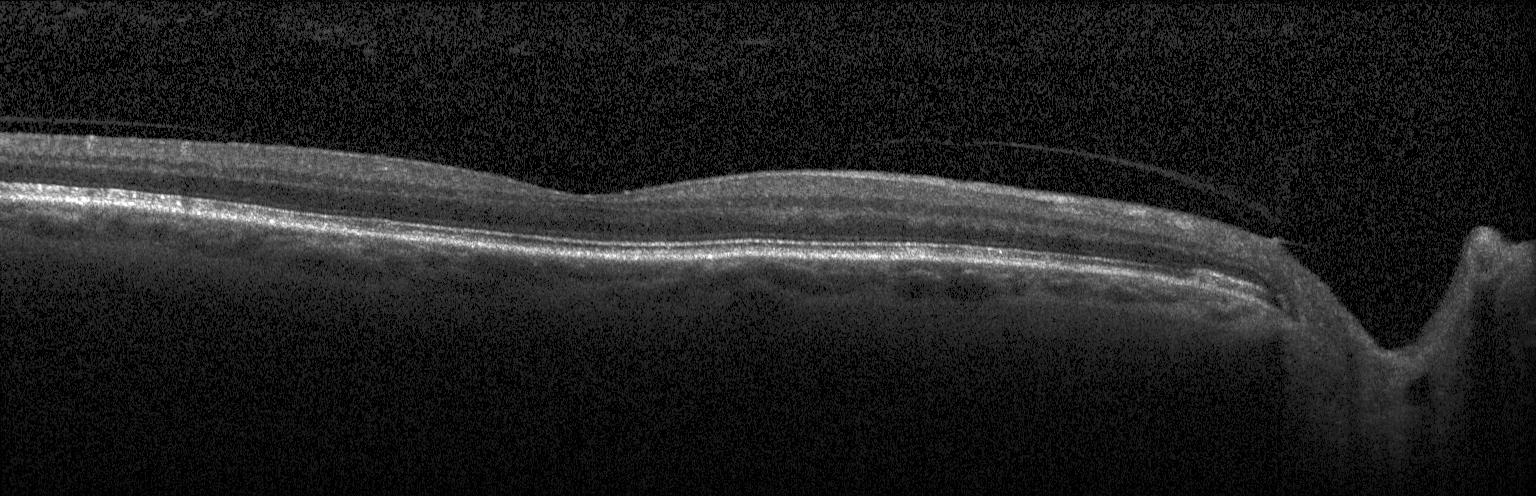
OCT finding: neither choroidal neovascularization, diabetic macular edema, nor drusen.